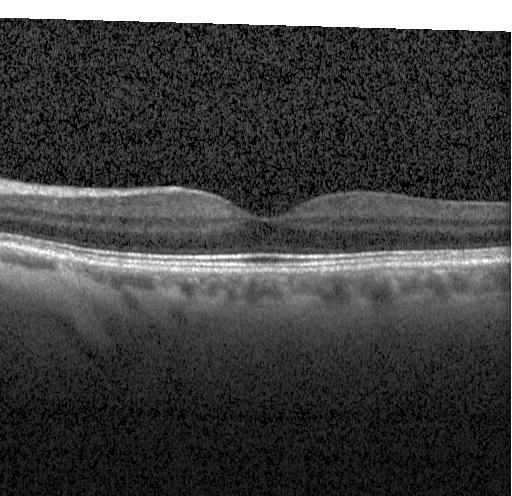

Macular OCT demonstrating no choroidal neovascularization, diabetic macular edema, or drusen.